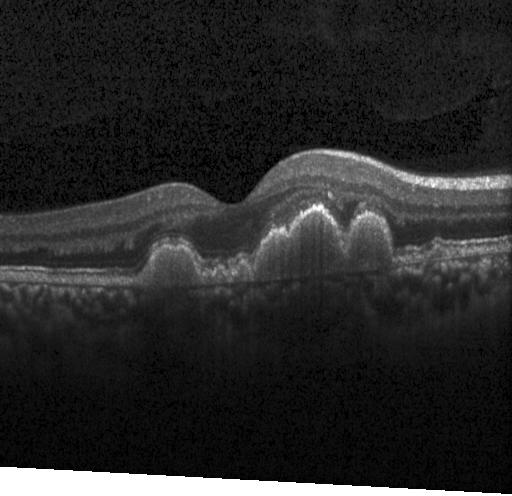

Retinal OCT B-scan — OCT finding: sub-RPE drusenoid deposits.